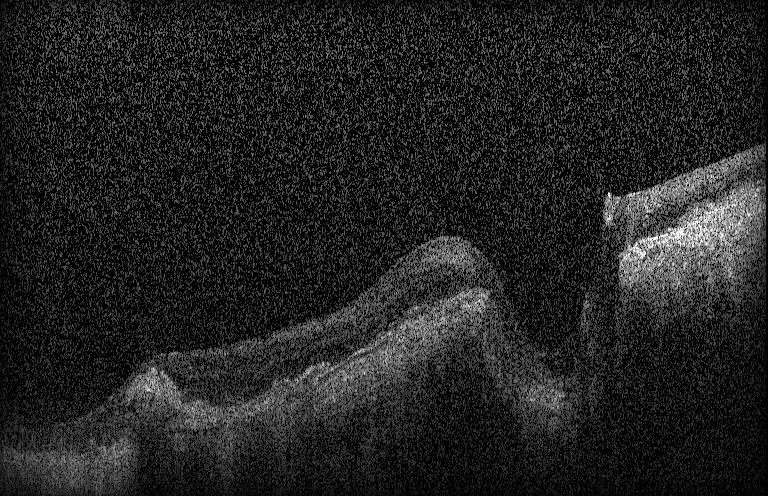

The scan shows choroidal neovascularization (CNV).